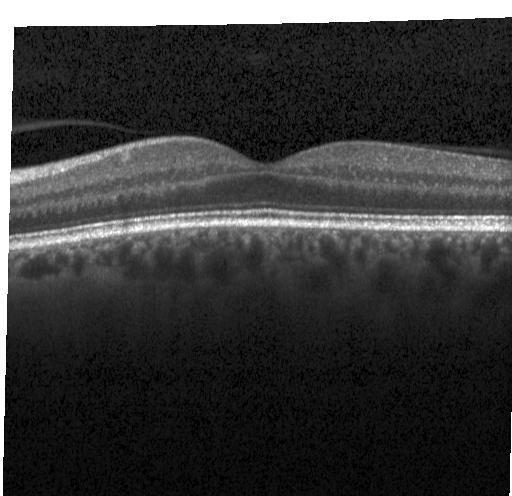

Diagnosis: no choroidal neovascularization, no diabetic macular edema, and no drusen.